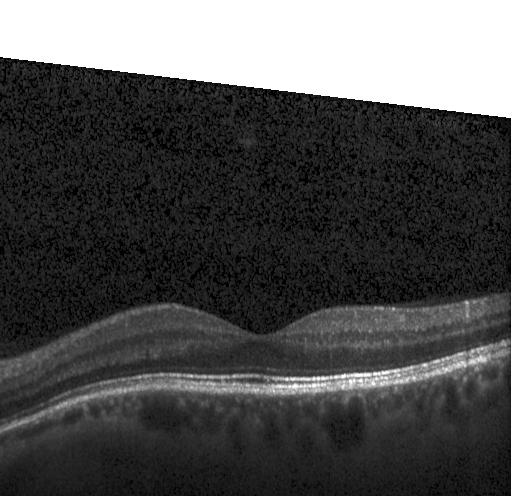

Macular OCT demonstrating no choroidal neovascularization, diabetic macular edema, or drusen.